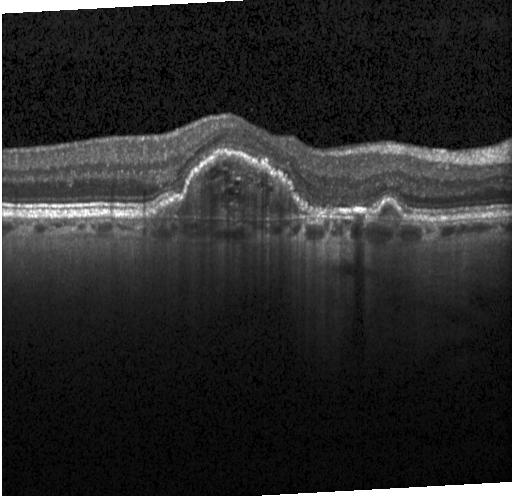
Impression: a choroidal neovascular membrane.